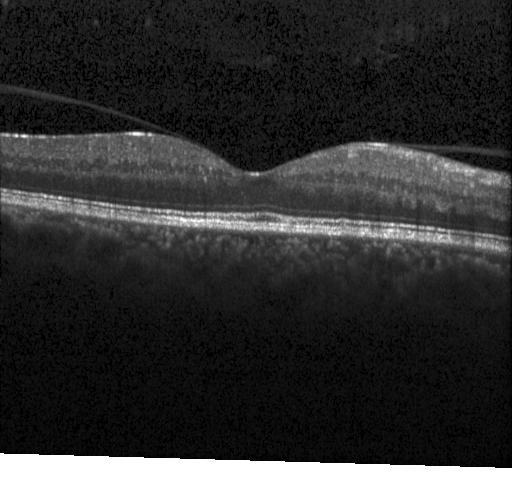

Optical coherence tomography scan
Diagnosis: no evidence of choroidal neovascularization, diabetic macular edema, or drusen.